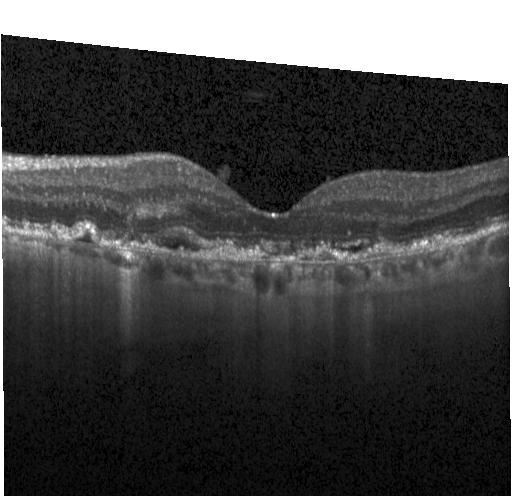 Optical coherence tomography B-scan. Finding: choroidal neovascularization.